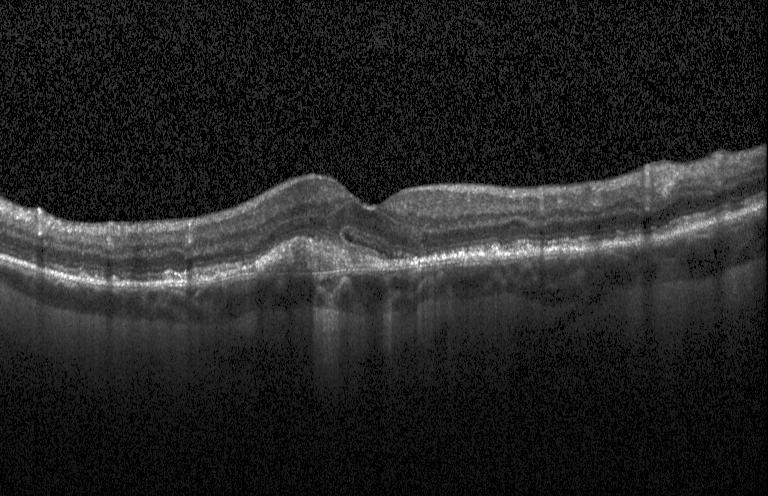

Retinal OCT cross-section, Heidelberg Spectralis OCT system, centered on the fovea, SD-OCT
Finding: a choroidal neovascular membrane.